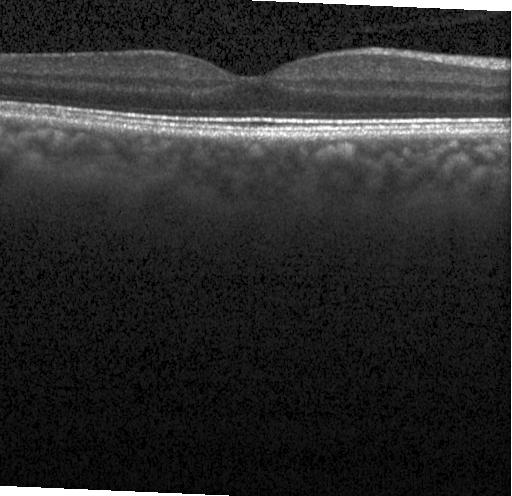
Finding: no evidence of choroidal neovascularization, diabetic macular edema, or drusen.